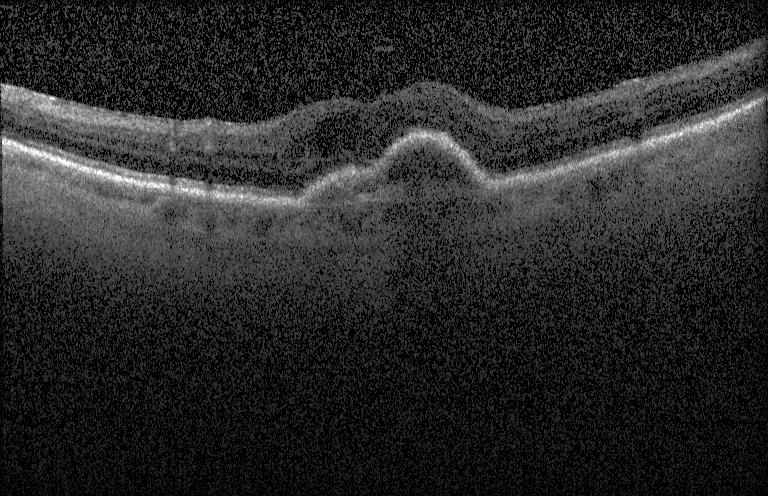

Retinal OCT B-scan
A choroidal neovascular membrane.